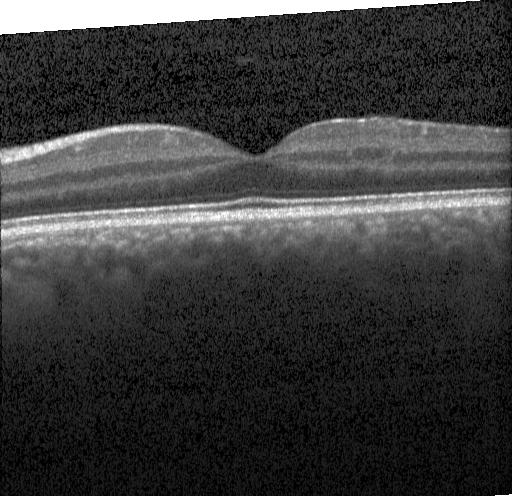 Dx: no evidence of CNV, DME, or drusen.